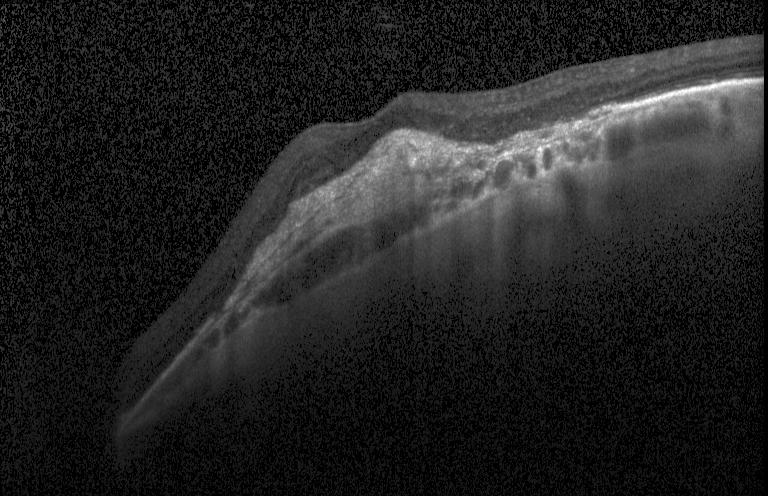 Spectral-domain OCT, retinal OCT cross-section, horizontal scan through the fovea
Impression: a choroidal neovascular membrane.